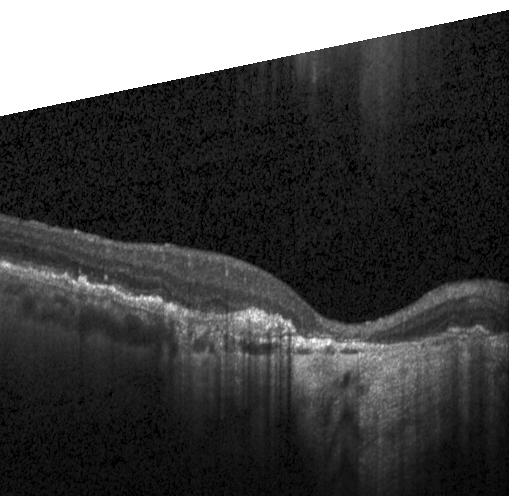
Retinal OCT cross-section showing CNV.